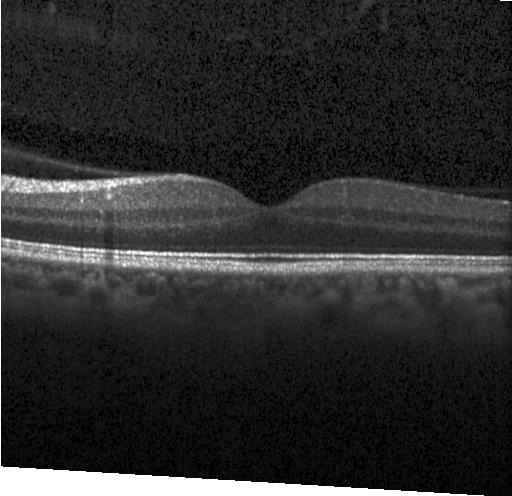

Diagnosis: neither choroidal neovascularization, diabetic macular edema, nor drusen.